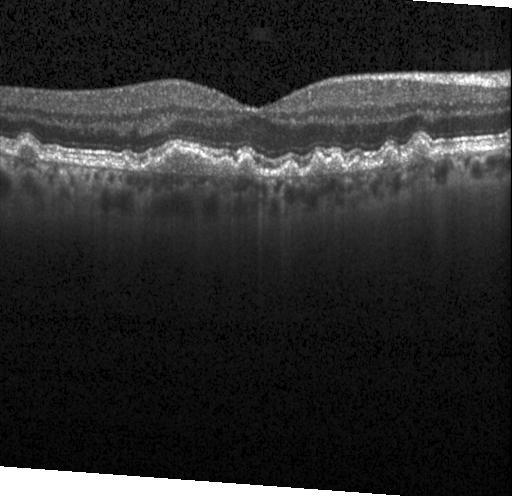
Optical coherence tomography scan; through the macula; Heidelberg Spectralis OCT system; spectral-domain OCT
Finding: multiple drusen.